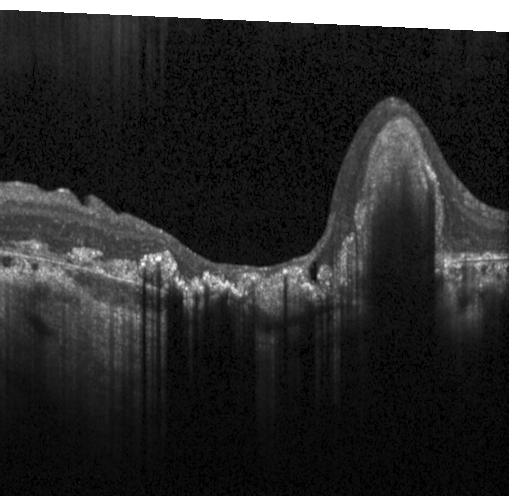

Optical coherence tomography scan. Spectral-domain OCT. Macular scan. Heidelberg Spectralis OCT system — Impression: a choroidal neovascular membrane.